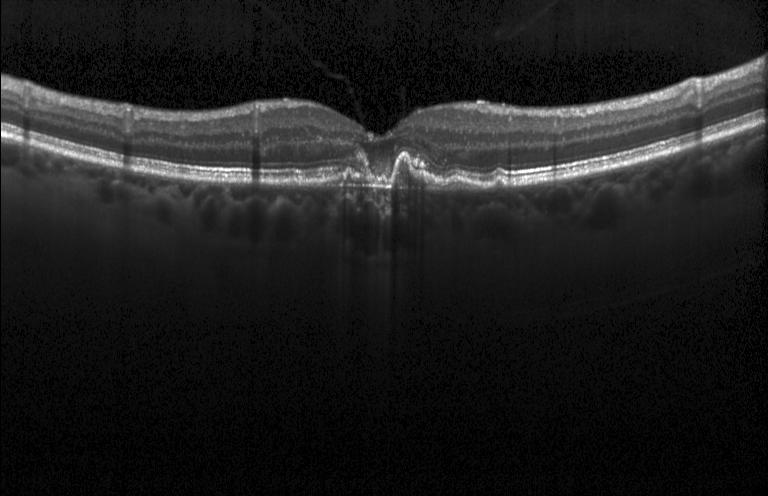 OCT line scan · spectral-domain optical coherence tomography · horizontal scan through the fovea
Assessment: choroidal neovascularization.